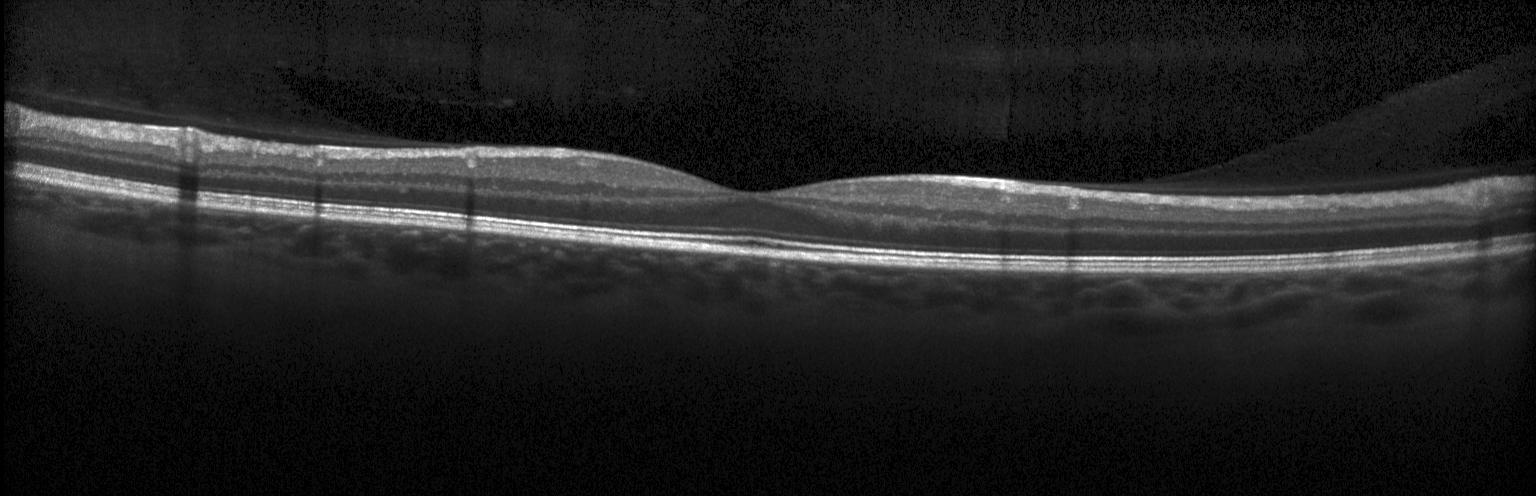 Dx: neither choroidal neovascularization, diabetic macular edema, nor drusen.